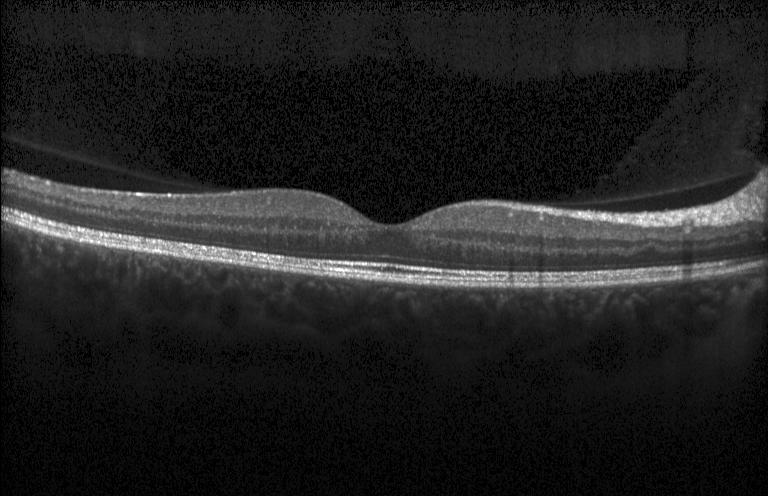 Finding: no choroidal neovascularization, no diabetic macular edema, and no drusen.